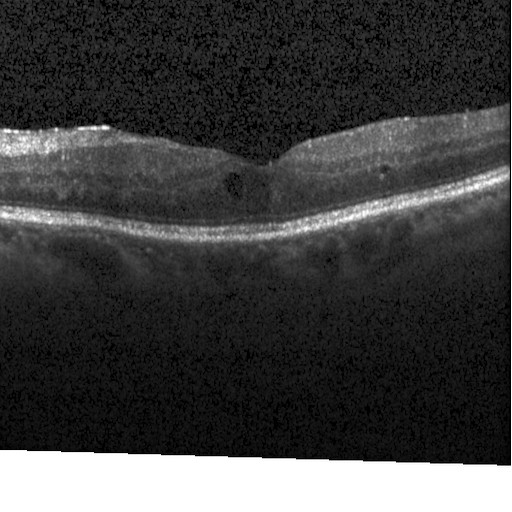
OCT finding: diabetic macular edema (DME).